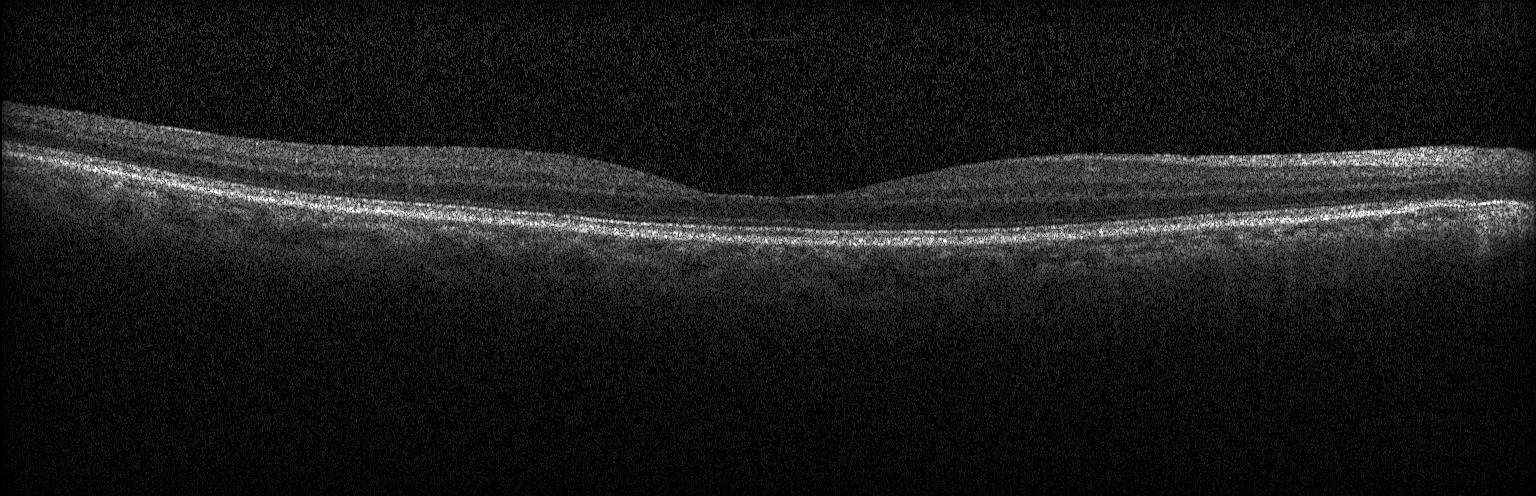

Dx: no CNV, DME, or drusen.